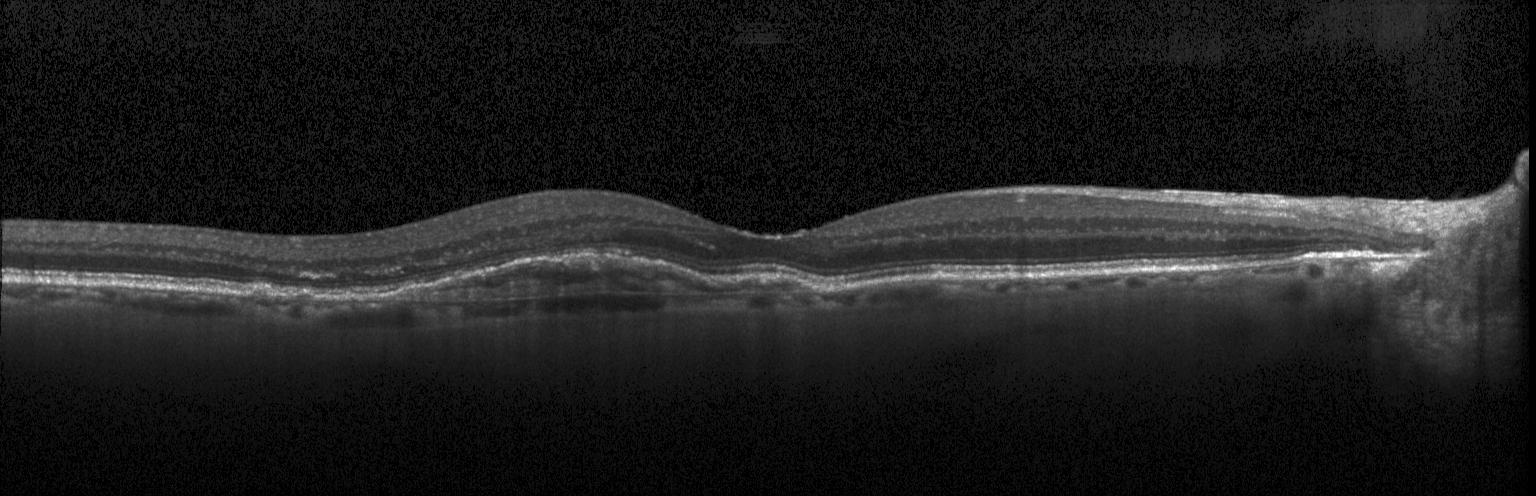 Impression: CNV.